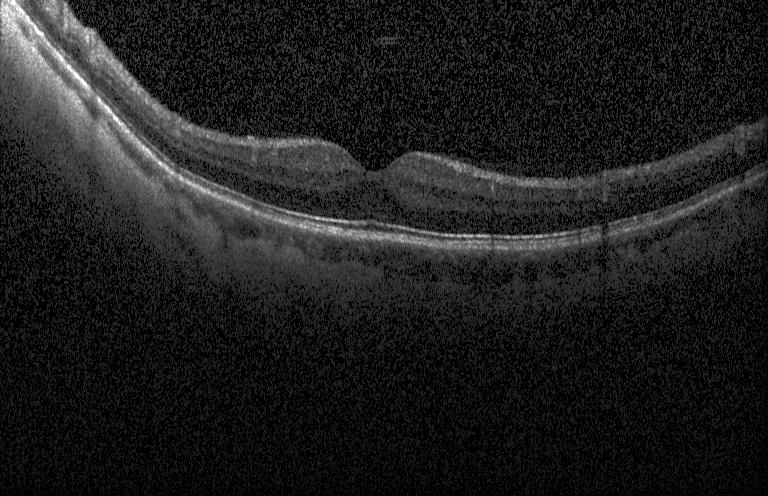

Optical coherence tomography scan
The scan shows neither choroidal neovascularization, diabetic macular edema, nor drusen.